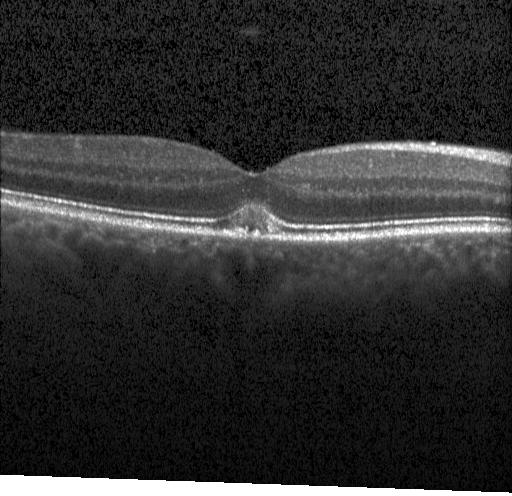 SD-OCT; instrument: Heidelberg Spectralis; optical coherence tomography scan.
Macular OCT: a choroidal neovascular membrane.